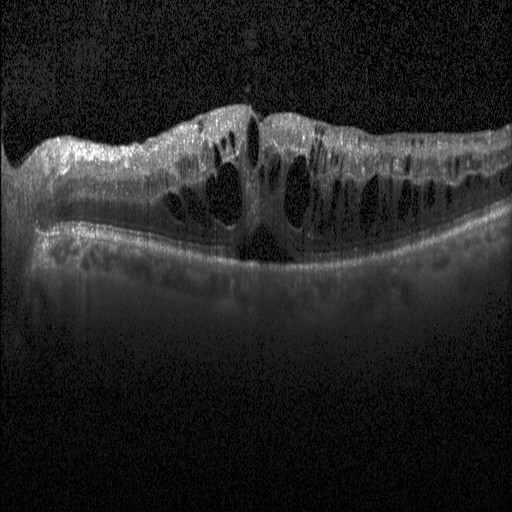

OCT B-scan · centered on the fovea · spectral-domain OCT · instrument: Heidelberg Spectralis — Finding: diabetic macular edema (DME).